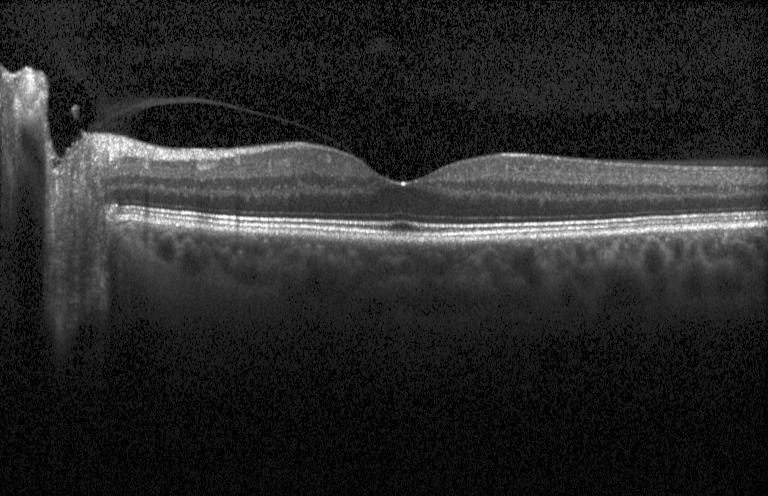
Spectral-domain OCT. Macular scan. Optical coherence tomography B-scan. Instrument: Heidelberg Spectralis.
Impression: no CNV, DME, or drusen.